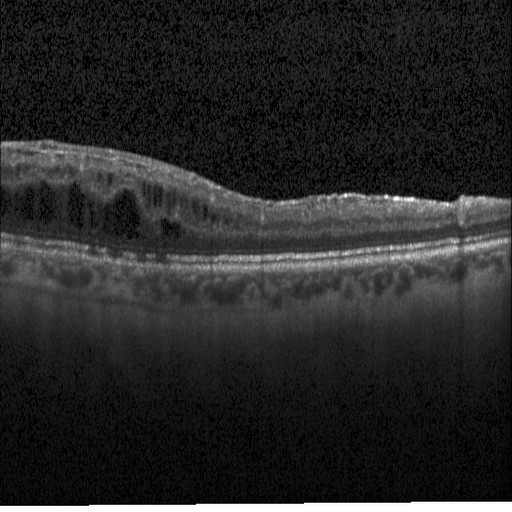
Macular scan · Heidelberg Spectralis · retinal OCT cross-section.
The scan shows diabetic macular edema.